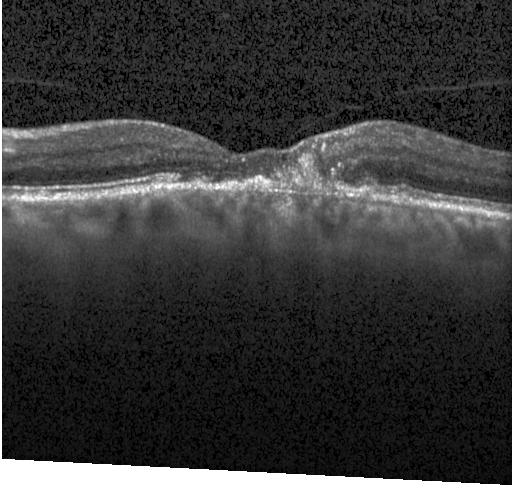 OCT finding: choroidal neovascularization (CNV).